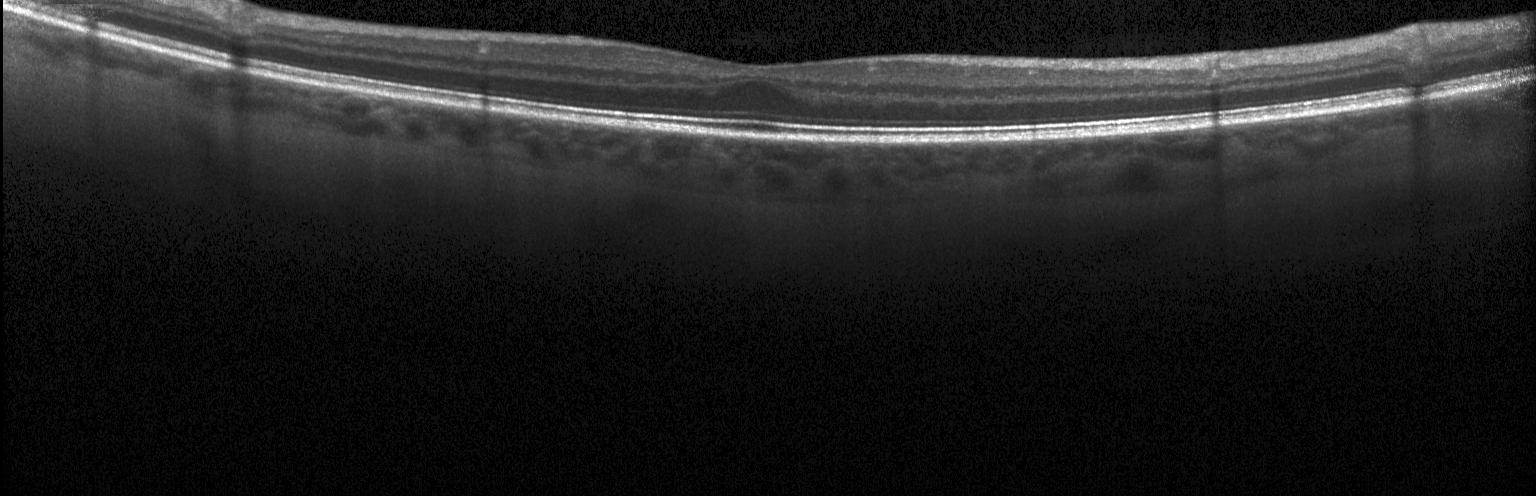 Horizontal scan through the fovea; retinal OCT cross-section; spectral-domain OCT.
Dx: no evidence of CNV, DME, or drusen.